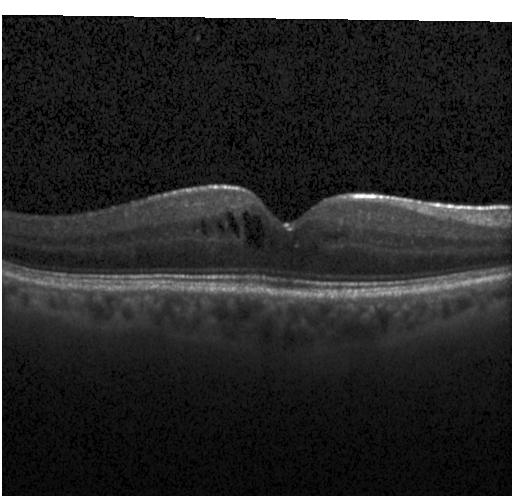 Diagnosis: diabetic macular edema.